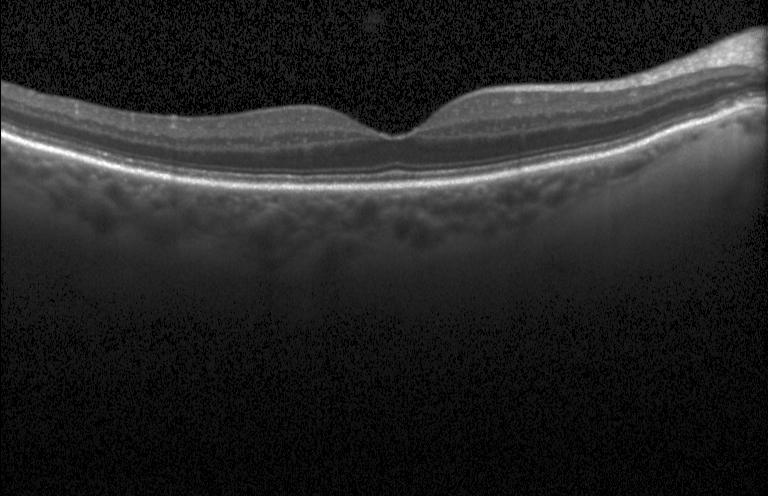
OCT finding: no evidence of CNV, DME, or drusen.